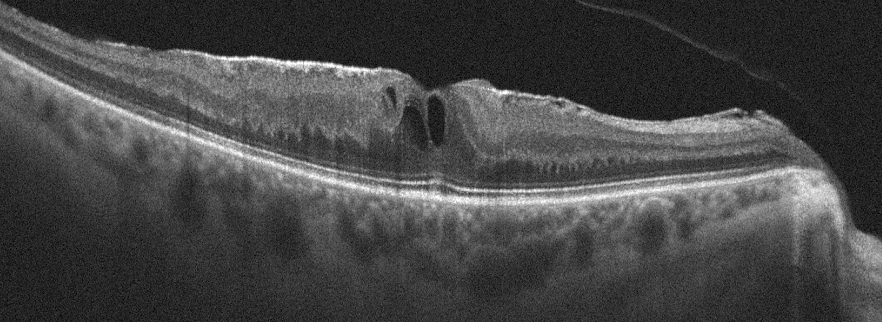

Retinal OCT cross-section. OD
OCT finding: ERM.